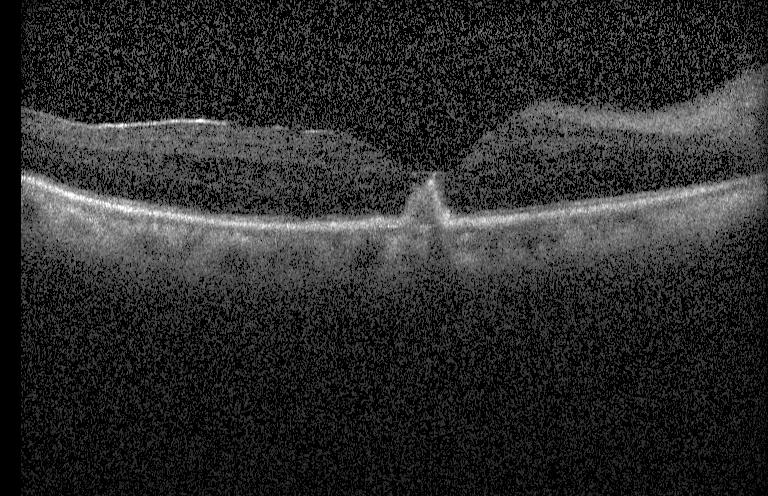

Centered on the fovea · retinal OCT B-scan · instrument: Heidelberg Spectralis.
Assessment: CNV.